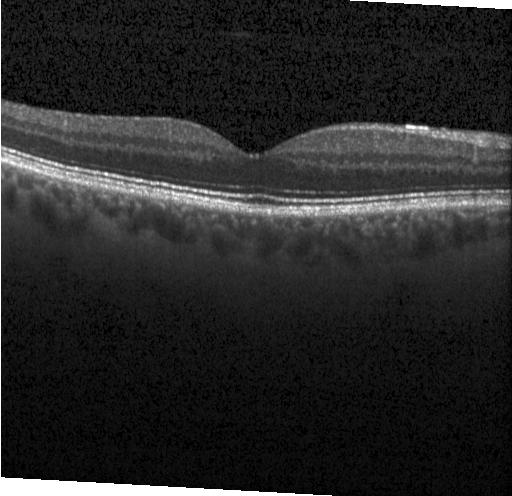

Optical coherence tomography B-scan; acquired on a Heidelberg Spectralis; fovea-centered; spectral-domain OCT
Impression: no choroidal neovascularization, diabetic macular edema, or drusen.